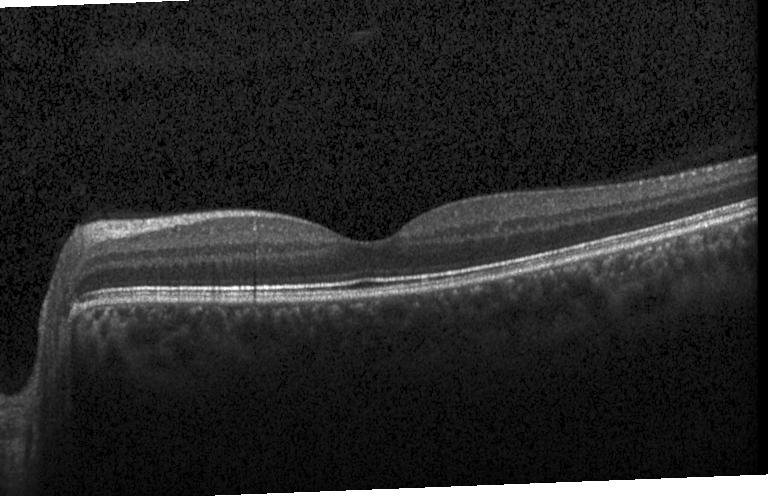

Macular scan, optical coherence tomography scan — Dx: no evidence of choroidal neovascularization, diabetic macular edema, or drusen.